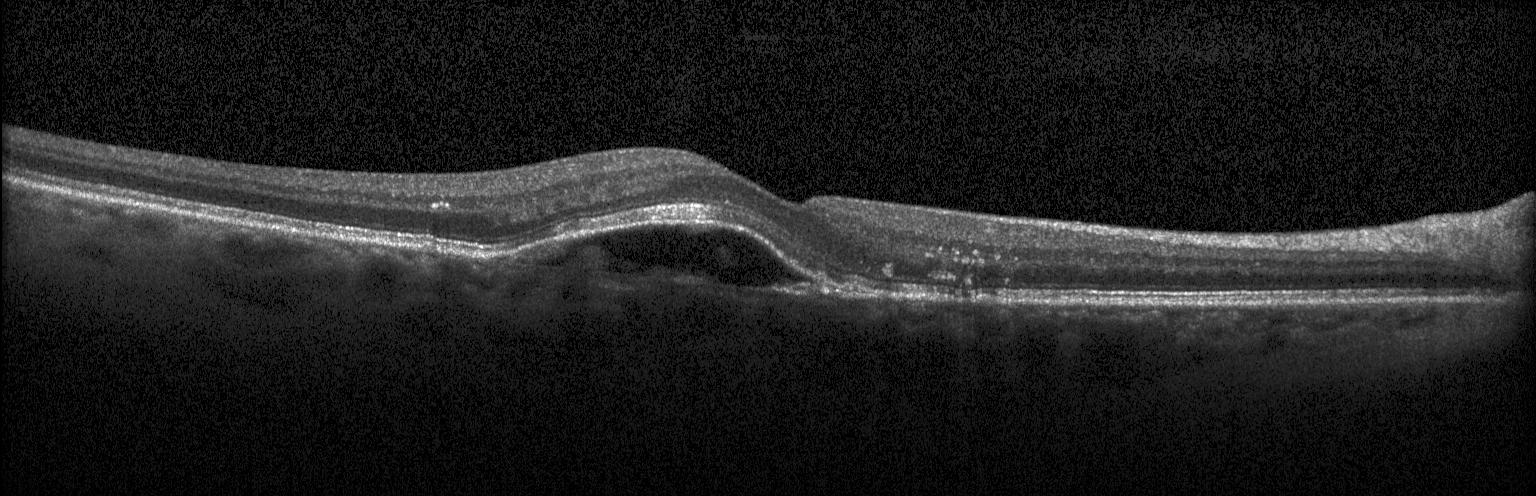

Finding: a choroidal neovascular membrane.